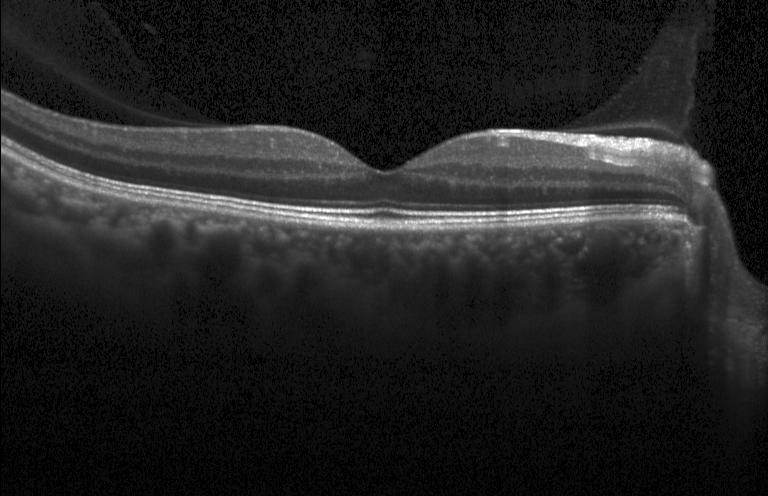 Spectral-domain optical coherence tomography; OCT B-scan.
No choroidal neovascularization, no diabetic macular edema, and no drusen.